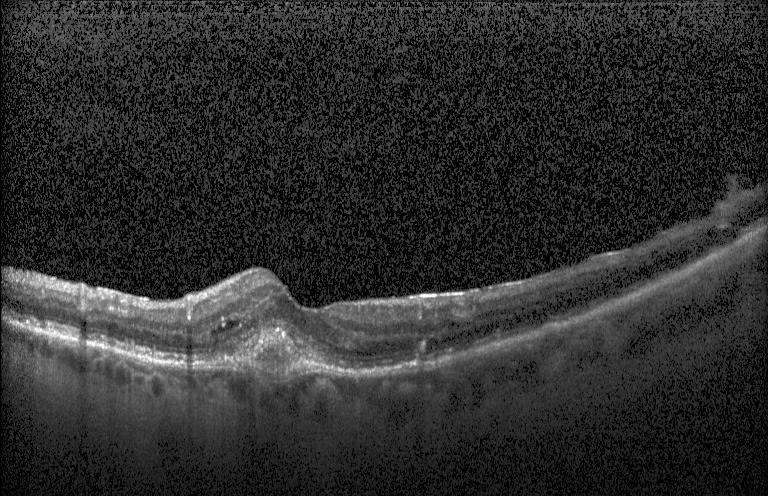

Retinal OCT cross-section showing choroidal neovascularization.